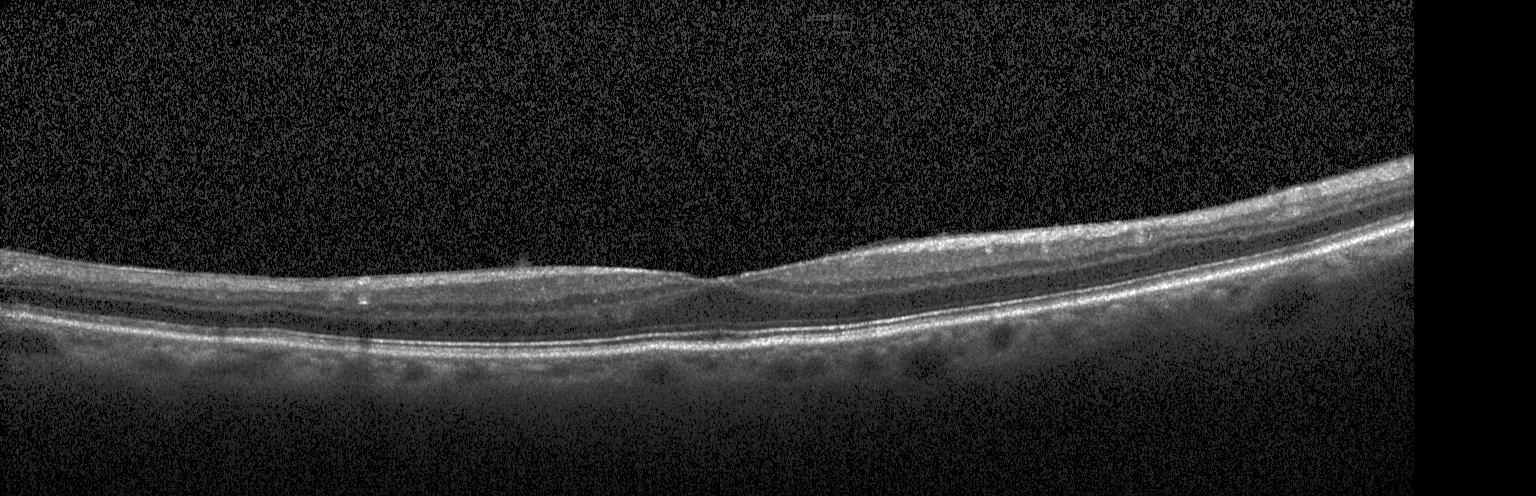
Retinal OCT cross-section showing neither choroidal neovascularization, diabetic macular edema, nor drusen.